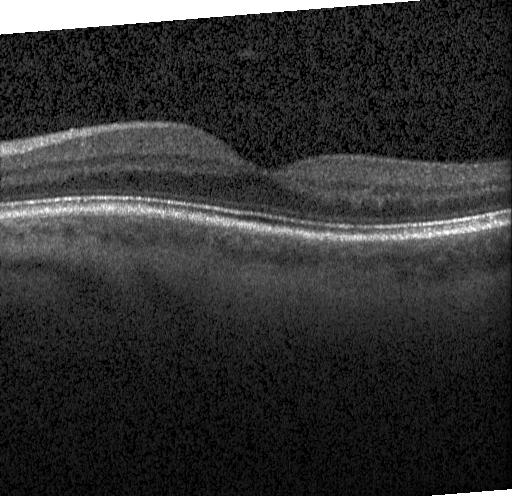

Spectral-domain OCT. Centered on the fovea. OCT line scan.
Finding: neither choroidal neovascularization, diabetic macular edema, nor drusen.